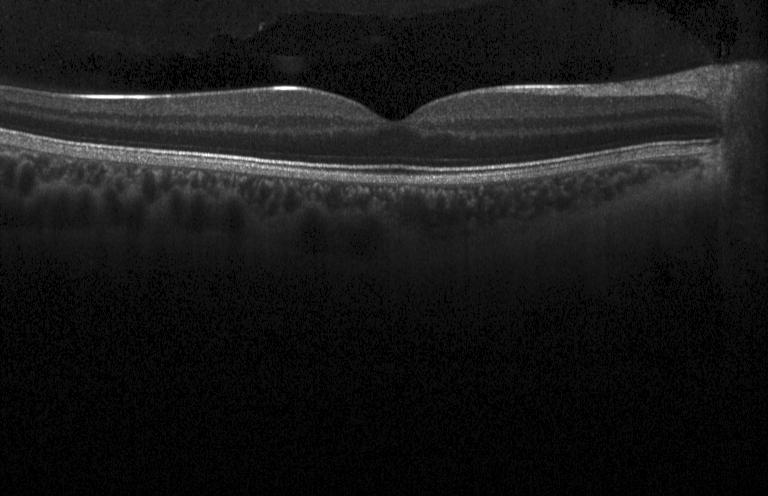 Finding: no CNV, DME, or drusen.